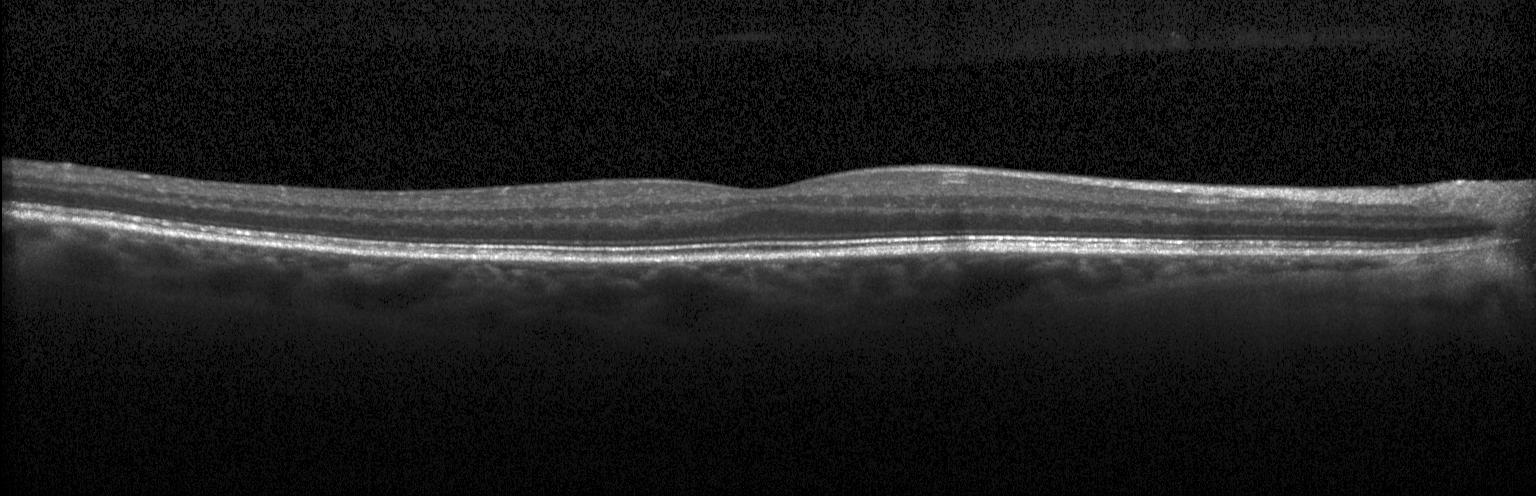 Heidelberg Spectralis. SD-OCT. Optical coherence tomography B-scan. Through the macula
Impression: no CNV, no DME, and no drusen.